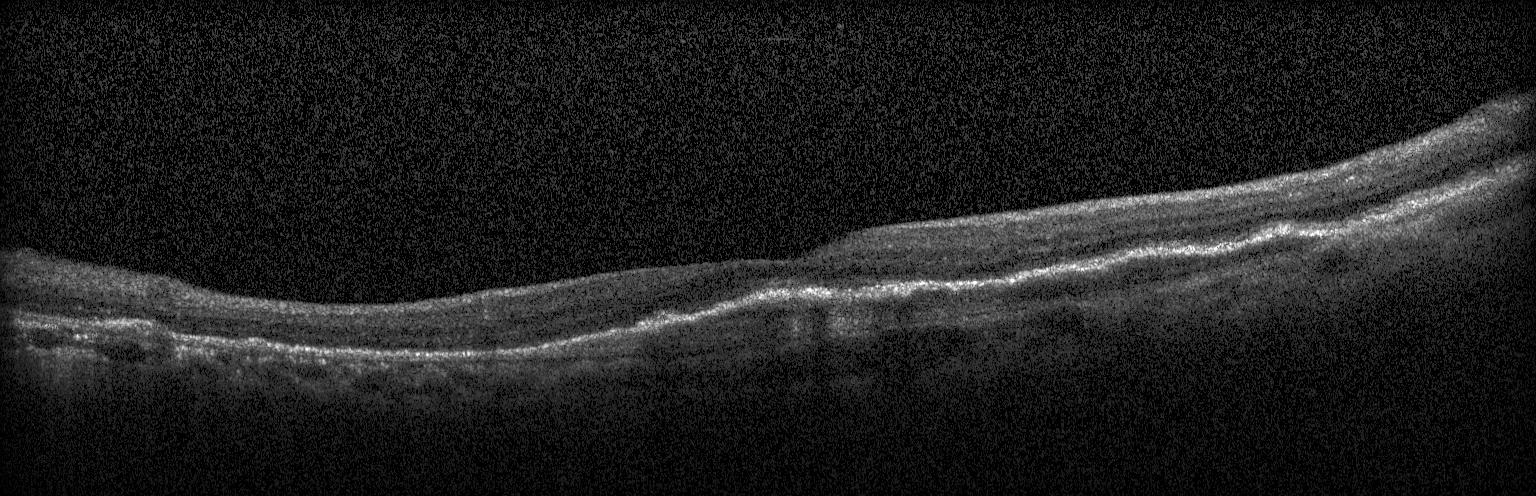 Optical coherence tomography scan. Diagnosis: a choroidal neovascular membrane.